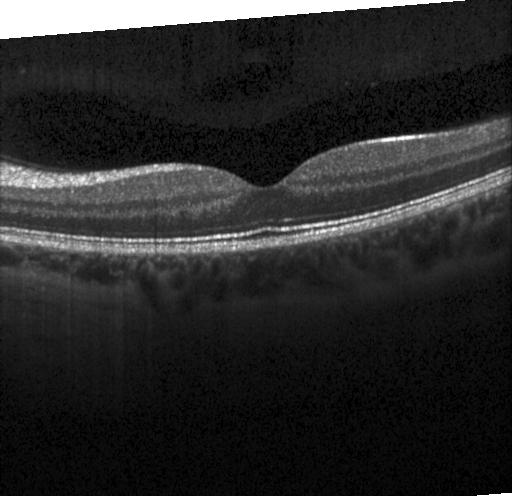

Retinal OCT B-scan — No choroidal neovascularization, no diabetic macular edema, and no drusen.